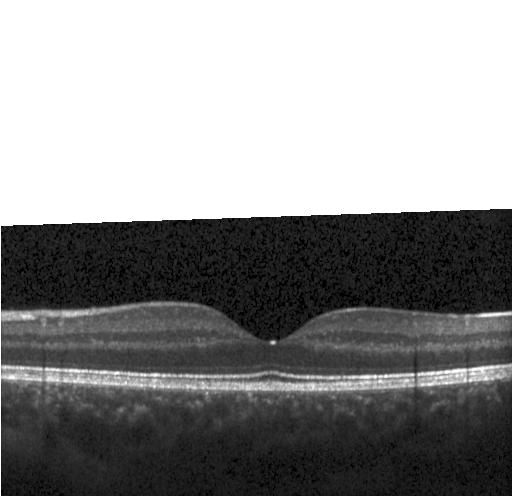

Assessment: no evidence of choroidal neovascularization, diabetic macular edema, or drusen.